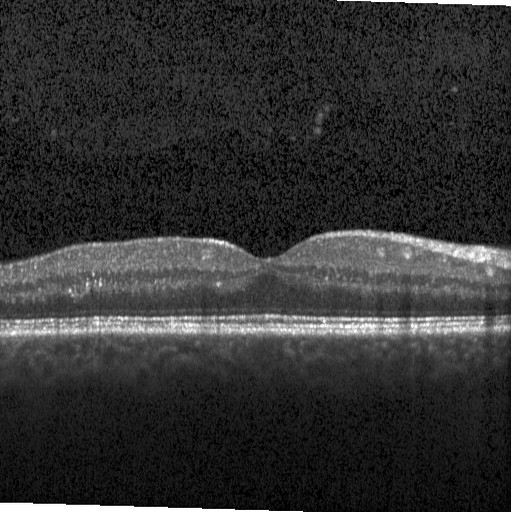

Macular scan. Spectral-domain optical coherence tomography. Instrument: Heidelberg Spectralis. Retinal OCT cross-section.
Finding: diabetic macular edema (DME).